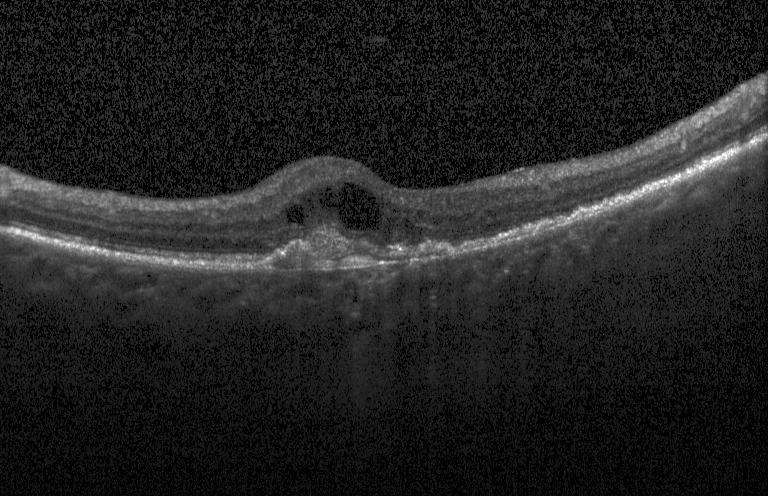

Macular scan. Retinal OCT B-scan
Assessment: a choroidal neovascular membrane.